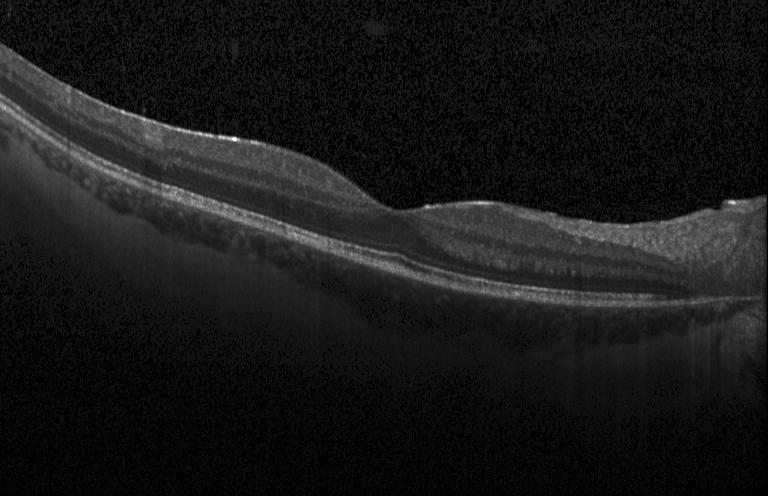 SD-OCT; macular scan; acquired on a Heidelberg Spectralis; OCT B-scan. Impression: no choroidal neovascularization, diabetic macular edema, or drusen.